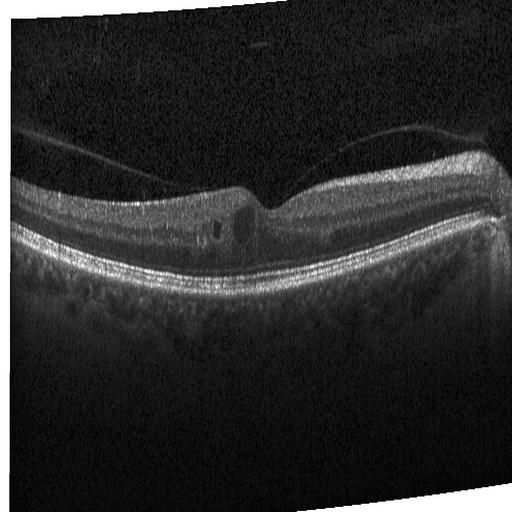 Fovea-centered; optical coherence tomography B-scan
Assessment: DME.